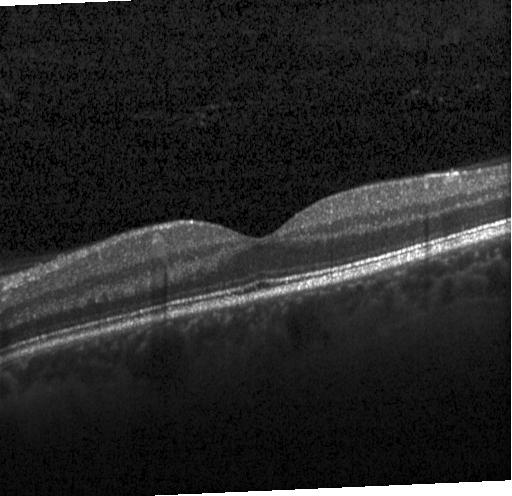
The scan shows no evidence of choroidal neovascularization, diabetic macular edema, or drusen.